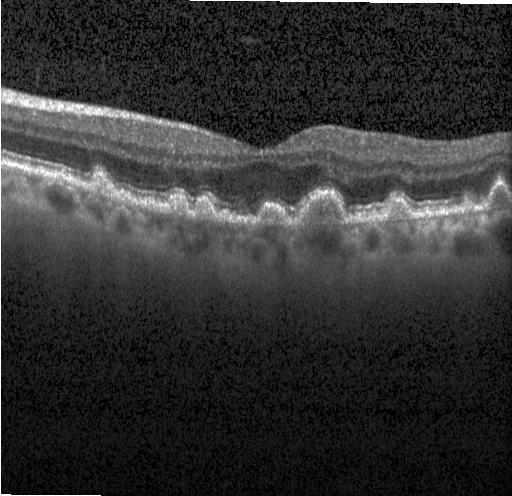

Centered on the fovea · acquired on a Heidelberg Spectralis · OCT line scan · spectral-domain optical coherence tomography. Impression: multiple drusen.